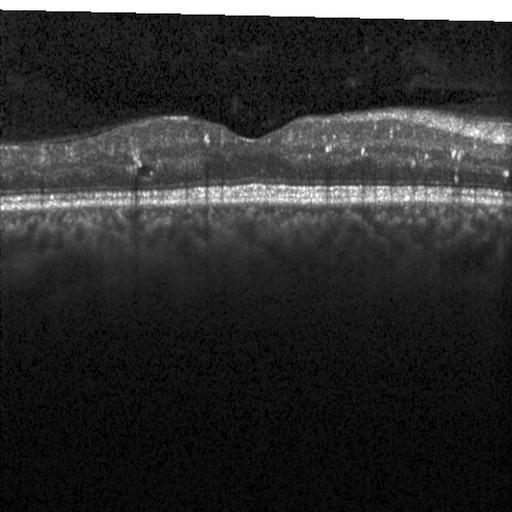

Spectral-domain OCT. OCT B-scan. Horizontal scan through the fovea.
Impression: diabetic macular edema (DME).